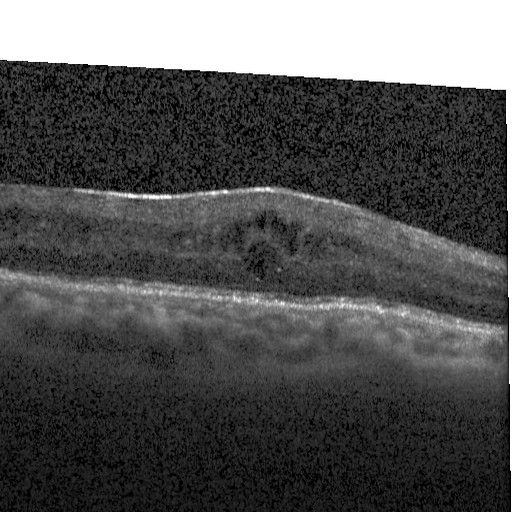 OCT B-scan. SD-OCT. Centered on the fovea
Assessment: diabetic macular edema (DME).